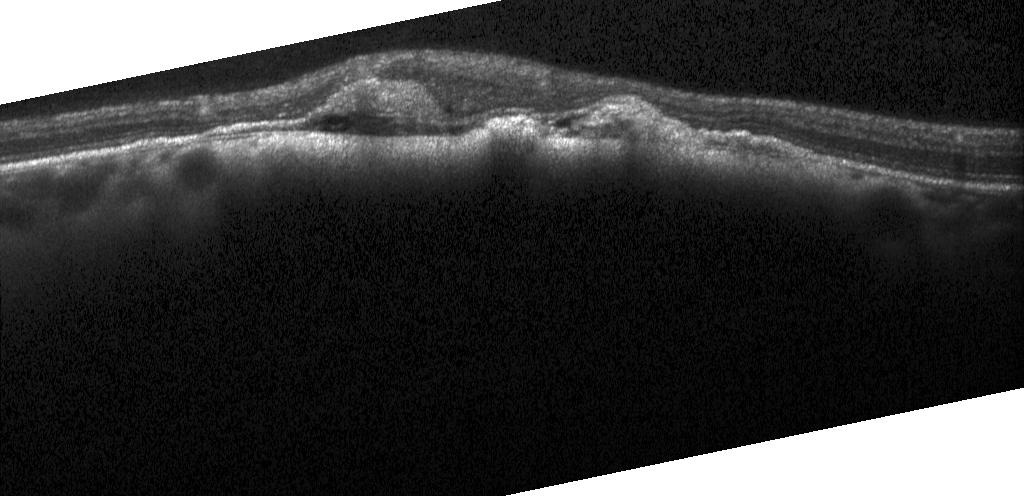

Retinal OCT B-scan
Impression: choroidal neovascularization.